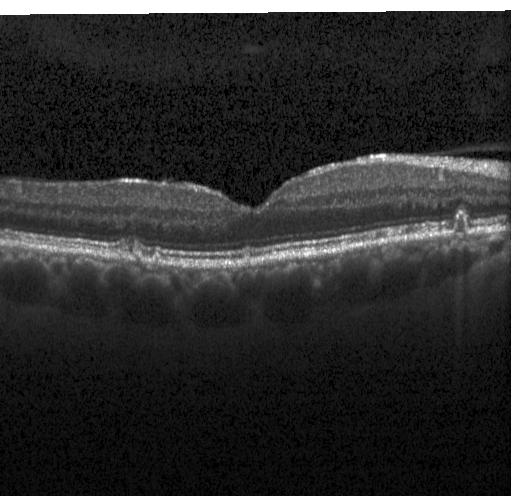

Diagnosis: sub-RPE drusenoid deposits.